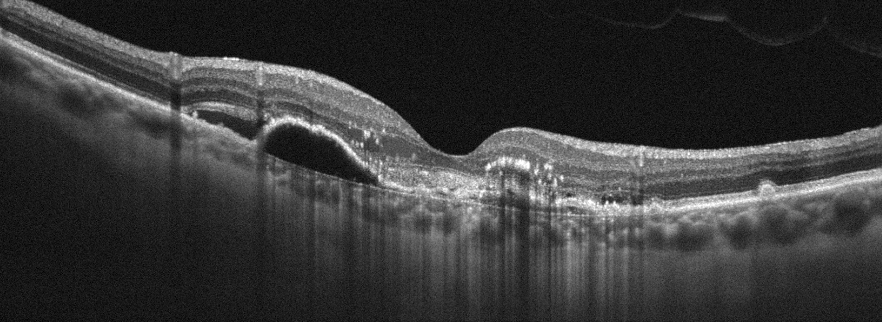 OCT B-scan
Finding: age-related macular degeneration.